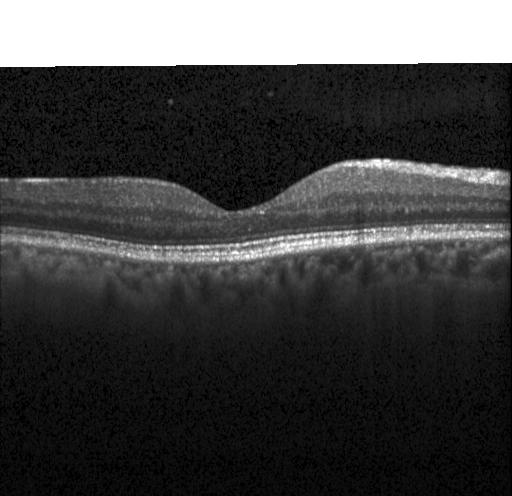
Retinal OCT cross-section
Macular OCT: no choroidal neovascularization, no diabetic macular edema, and no drusen.